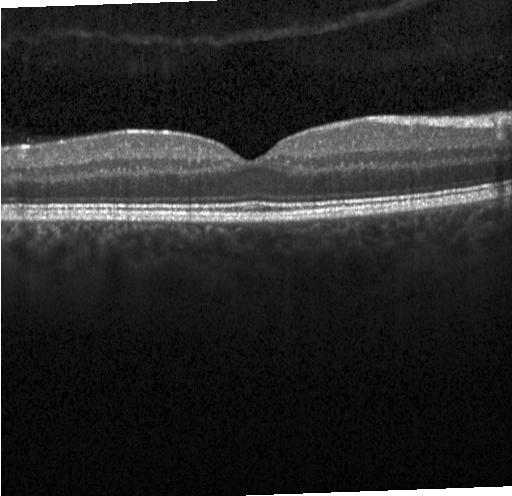 Impression: no choroidal neovascularization, no diabetic macular edema, and no drusen.